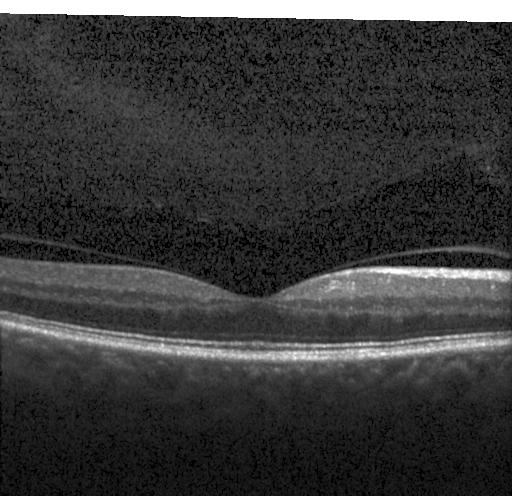
Instrument: Heidelberg Spectralis, retinal OCT B-scan, through the macula, spectral-domain OCT. The scan shows no evidence of choroidal neovascularization, diabetic macular edema, or drusen.